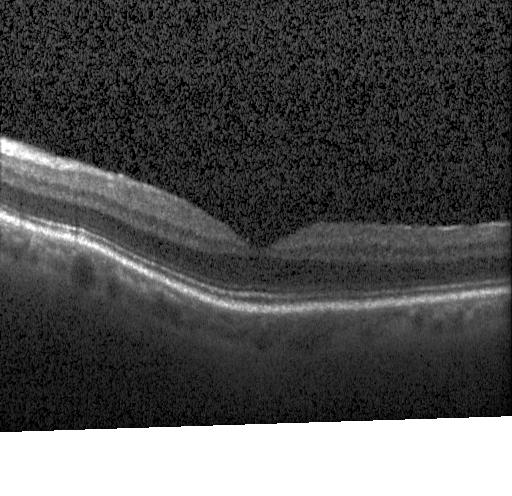
Through the macula; OCT line scan; spectral-domain OCT; Heidelberg Spectralis OCT system
Impression: neither choroidal neovascularization, diabetic macular edema, nor drusen.